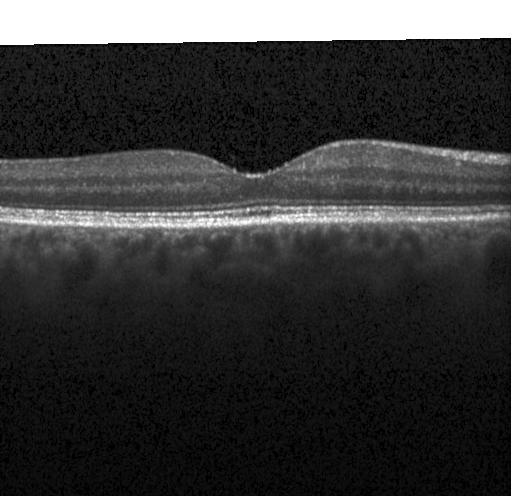

Dx: neither CNV, DME, nor drusen.